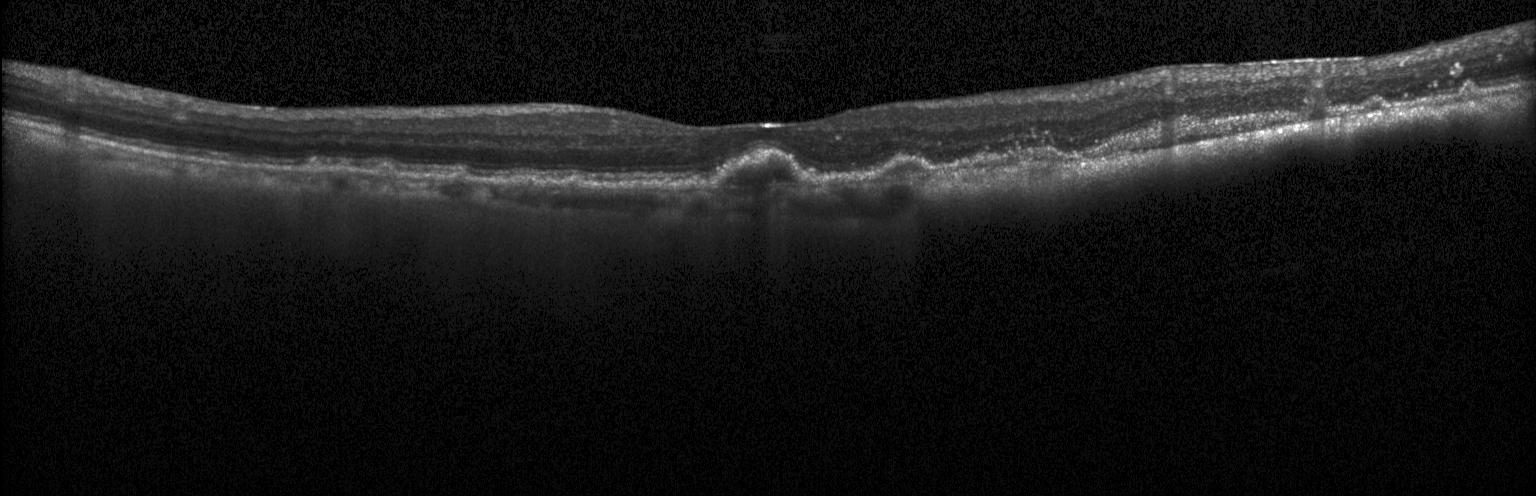

Dx: CNV.